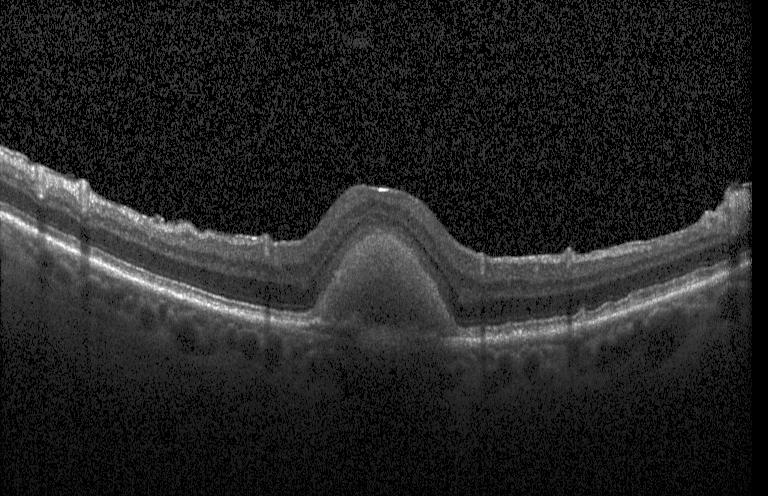
Macular scan. OCT B-scan. SD-OCT.
Dx: choroidal neovascularization (CNV).